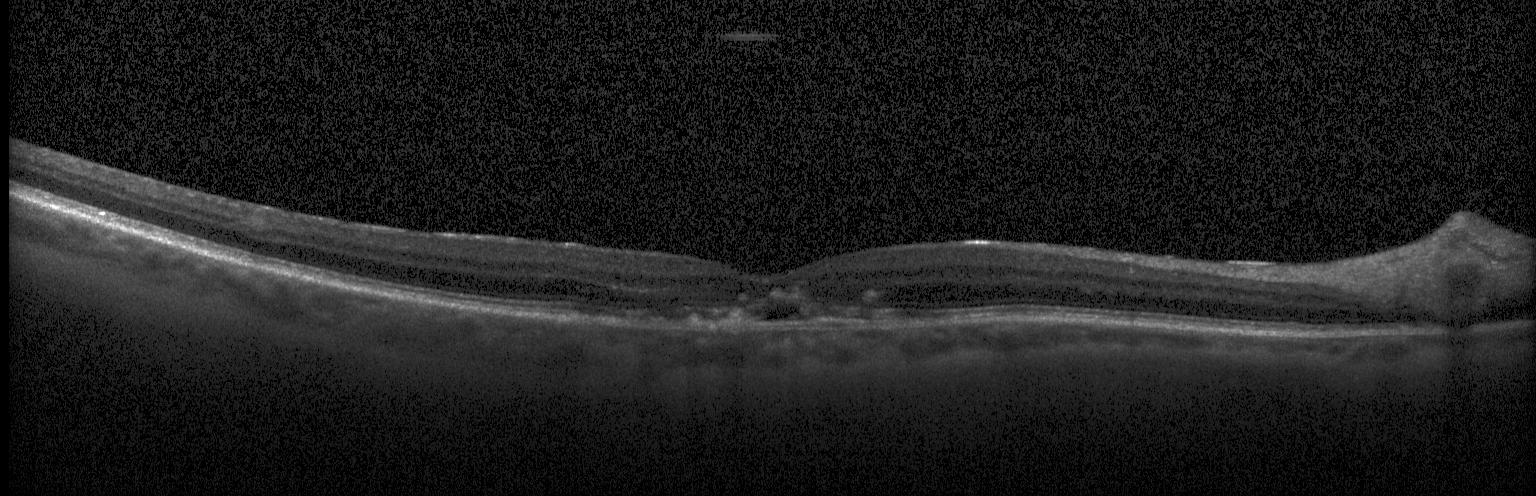

A choroidal neovascular membrane.